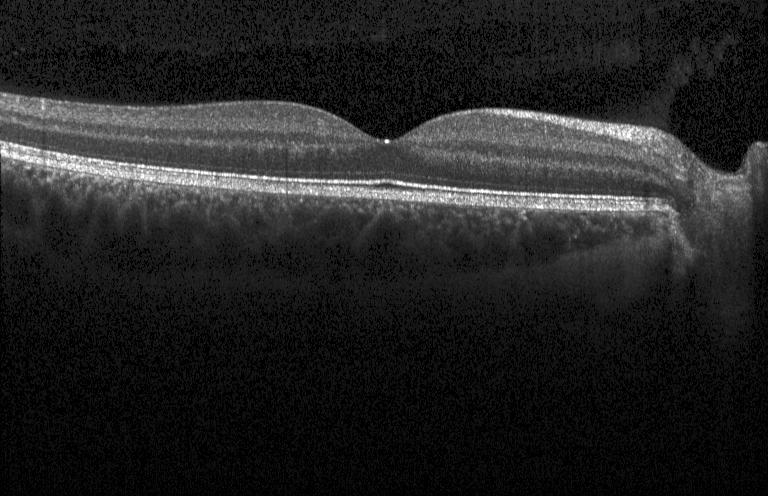

Finding: neither CNV, DME, nor drusen.